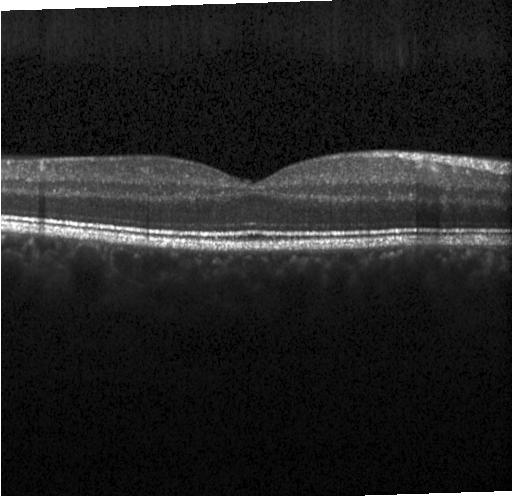
SD-OCT · Heidelberg Spectralis OCT system · optical coherence tomography scan.
Impression: no choroidal neovascularization, no diabetic macular edema, and no drusen.